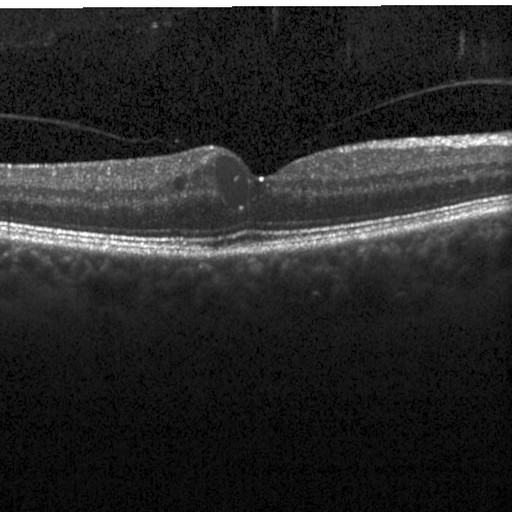

Spectral-domain OCT · optical coherence tomography scan. Diabetic macular edema (DME).